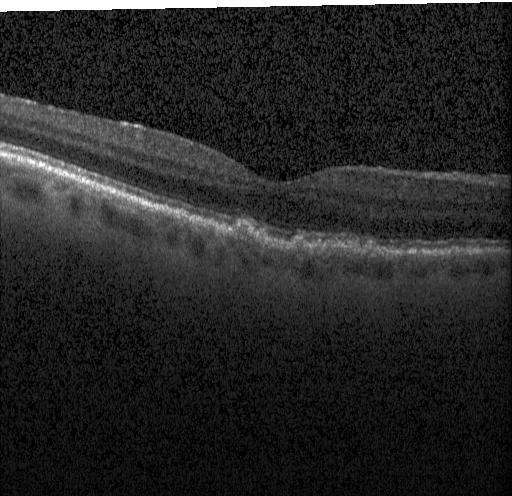
Impression: drusen.